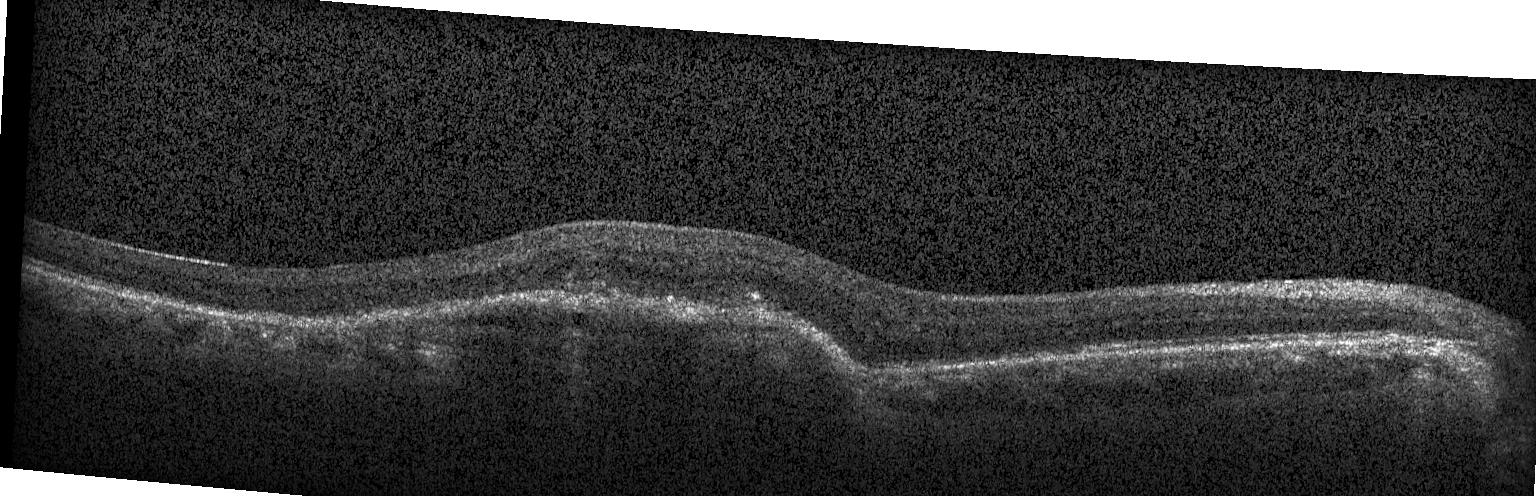
OCT B-scan. Spectral-domain optical coherence tomography. Acquired on a Heidelberg Spectralis
This B-scan demonstrates choroidal neovascularization (CNV).